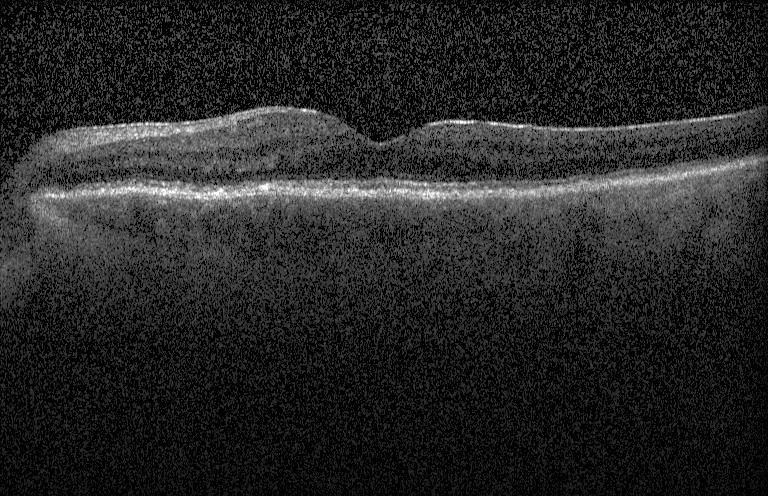 Spectral-domain OCT. Retinal OCT B-scan. Instrument: Heidelberg Spectralis — Finding: neither choroidal neovascularization, diabetic macular edema, nor drusen.